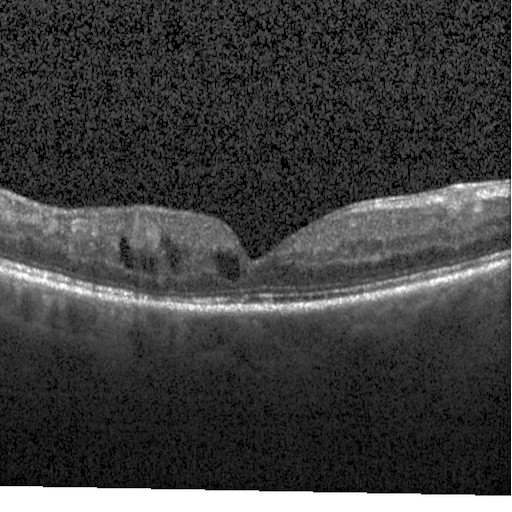 OCT B-scan showing diabetic macular edema.